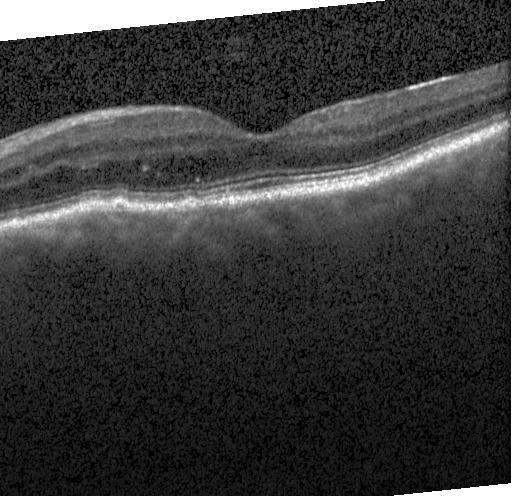

Through the macula · retinal OCT cross-section · spectral-domain optical coherence tomography · instrument: Heidelberg Spectralis
Diagnosis: DME.